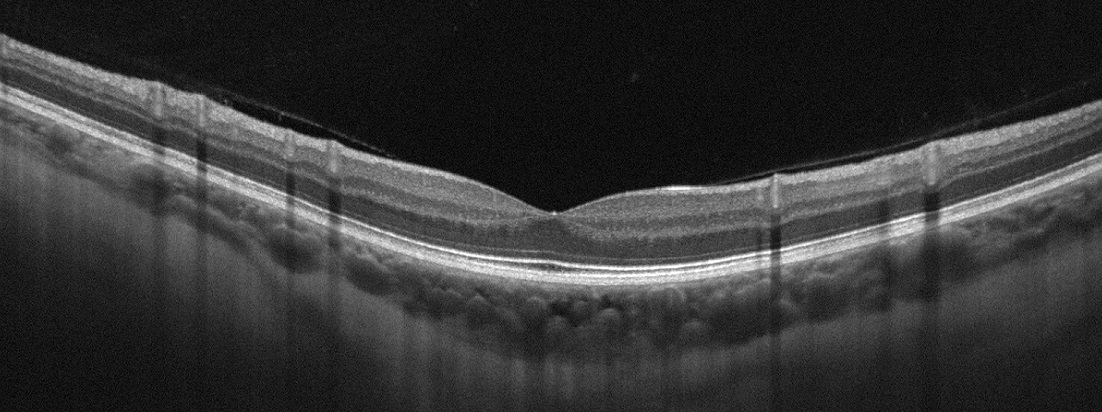

Assessment: no AMD, DME, ERM, RAO, RVO, or VID.